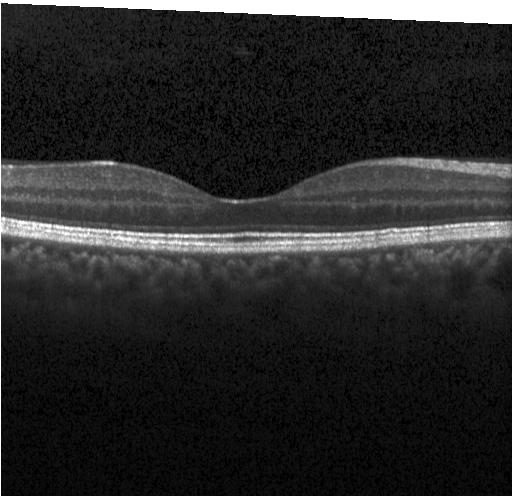
Instrument: Heidelberg Spectralis; OCT B-scan; spectral-domain optical coherence tomography.
Diagnosis: neither choroidal neovascularization, diabetic macular edema, nor drusen.